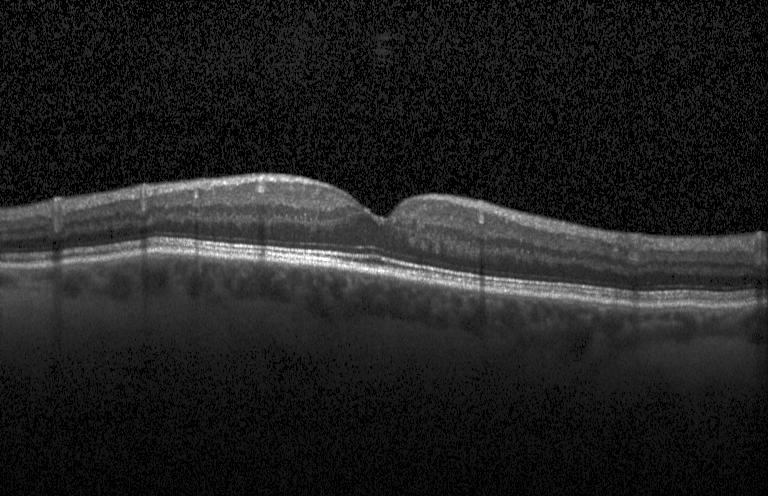 Macular OCT demonstrating no CNV, no DME, and no drusen.